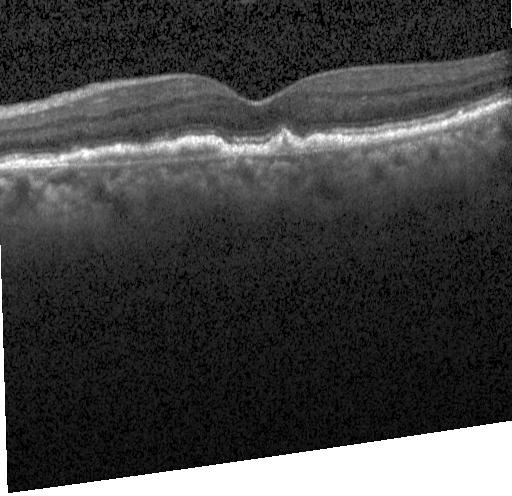
Optical coherence tomography scan; Heidelberg Spectralis; fovea-centered. Finding: a choroidal neovascular membrane.